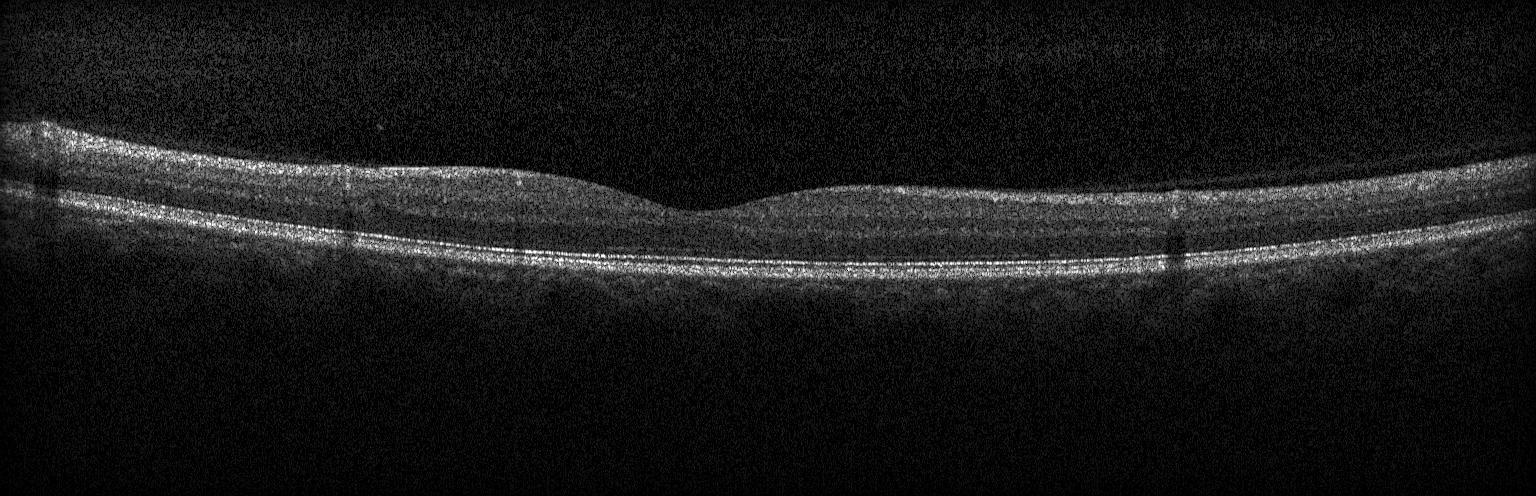 Spectral-domain OCT B-scan: neither choroidal neovascularization, diabetic macular edema, nor drusen.